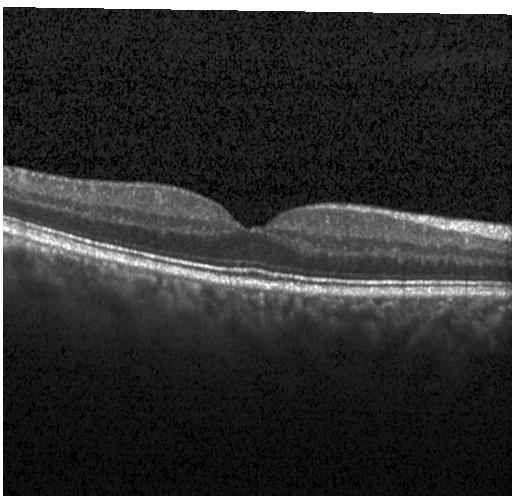 OCT finding: no evidence of CNV, DME, or drusen.